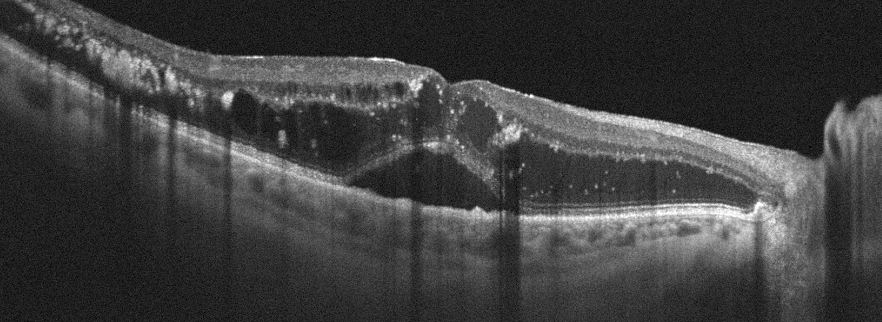 OD · Optovue Avanti RTVue XR · optical coherence tomography scan. The scan shows RVO.